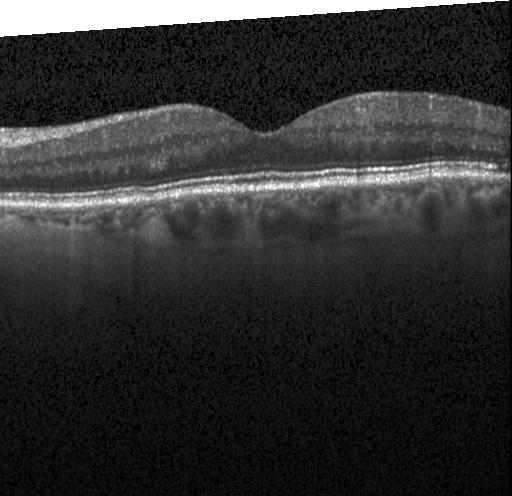 Optical coherence tomography scan. Spectral-domain optical coherence tomography. Heidelberg Spectralis — Impression: no choroidal neovascularization, diabetic macular edema, or drusen.